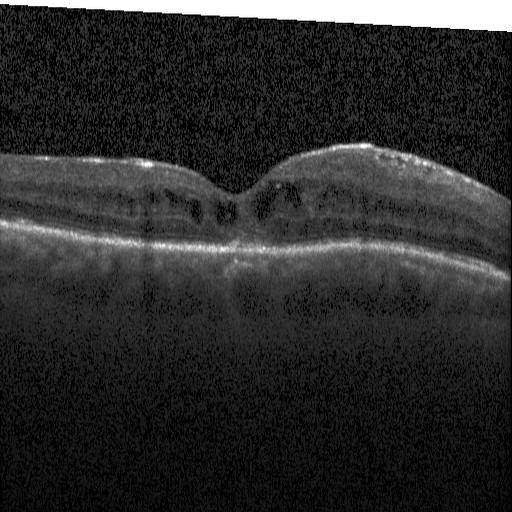

Retinal OCT B-scan.
This B-scan demonstrates DME.